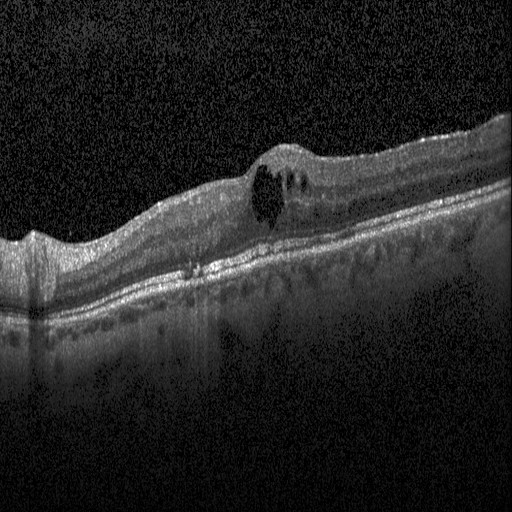

Horizontal scan through the fovea · Heidelberg Spectralis OCT system · retinal OCT B-scan
Macular OCT: diabetic macular edema.